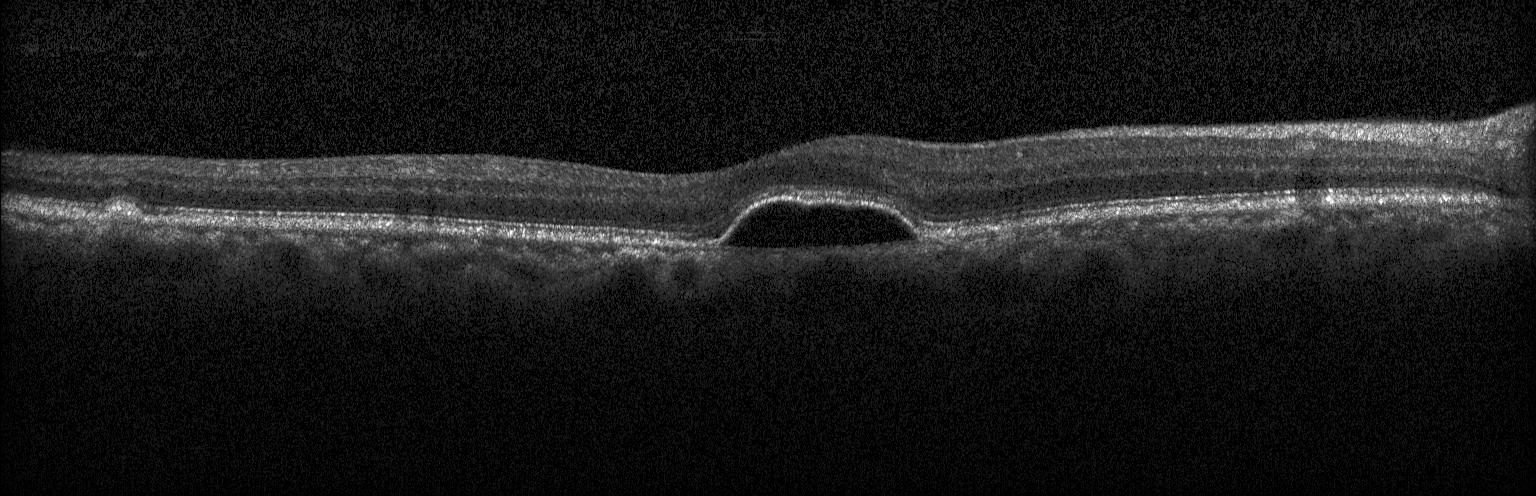 Fovea-centered. Heidelberg Spectralis. SD-OCT. OCT line scan.
Diagnosis: a choroidal neovascular membrane.